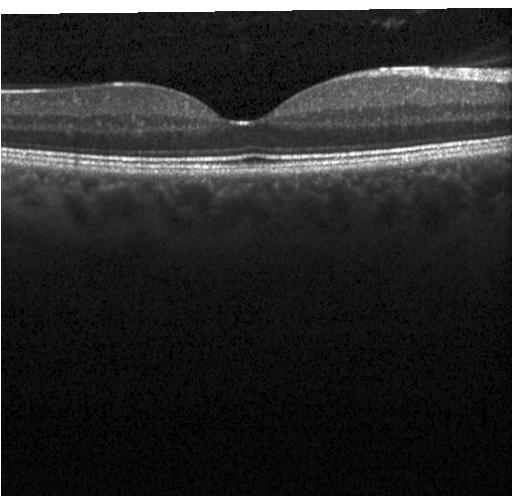
OCT finding: no evidence of choroidal neovascularization, diabetic macular edema, or drusen.